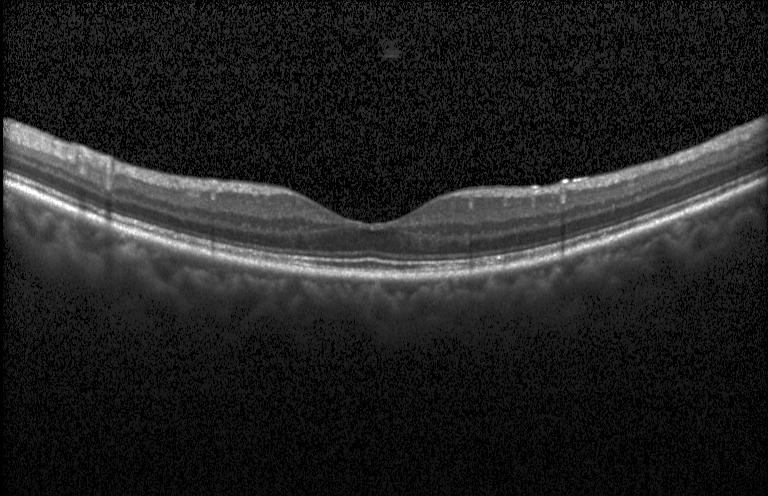 Impression: no evidence of CNV, DME, or drusen.